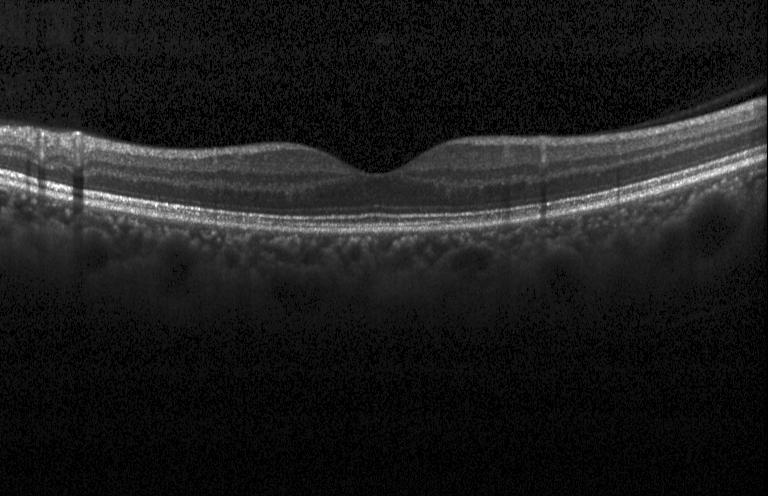

Through the macula; optical coherence tomography scan; SD-OCT.
OCT finding: no evidence of CNV, DME, or drusen.